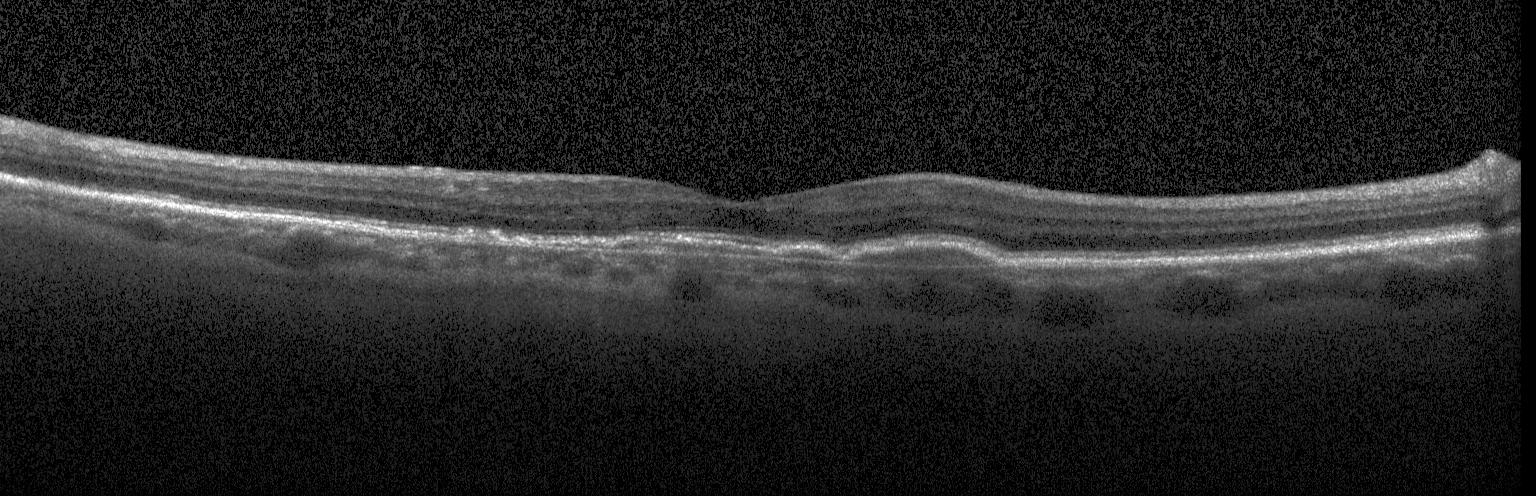 Finding: a choroidal neovascular membrane.